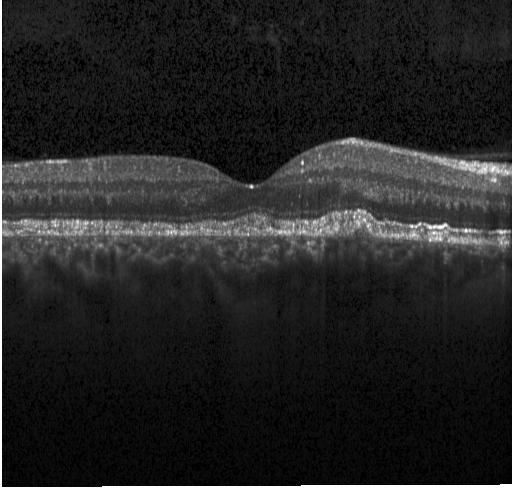

Horizontal scan through the fovea; spectral-domain OCT; OCT B-scan — Macular OCT: drusen.